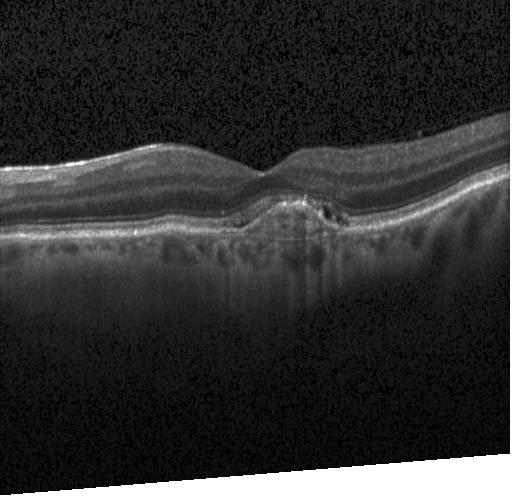 Acquired on a Heidelberg Spectralis · optical coherence tomography scan
Impression: choroidal neovascularization (CNV).